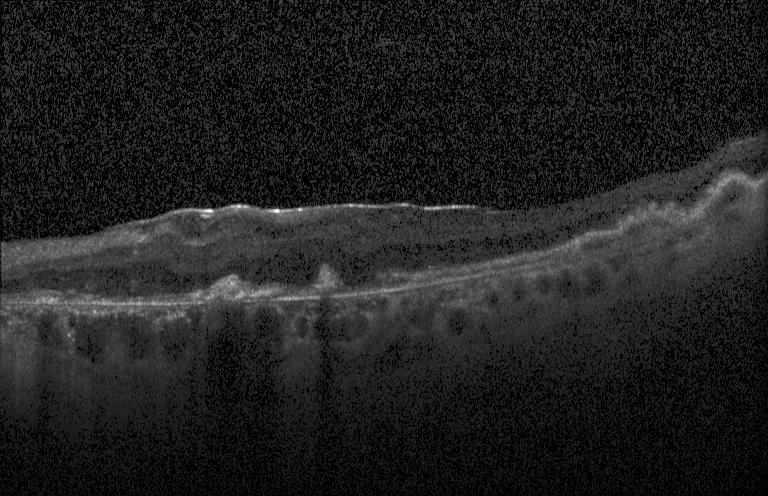

Optical coherence tomography scan · spectral-domain optical coherence tomography · Heidelberg Spectralis — Dx: CNV.